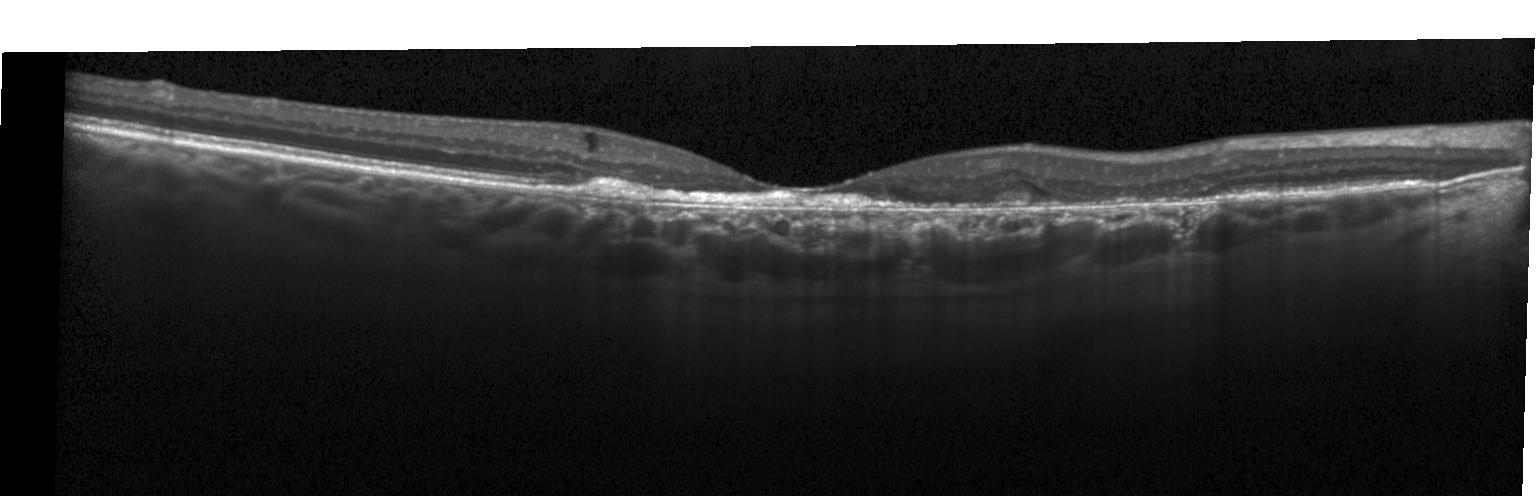
Macular OCT: a choroidal neovascular membrane.